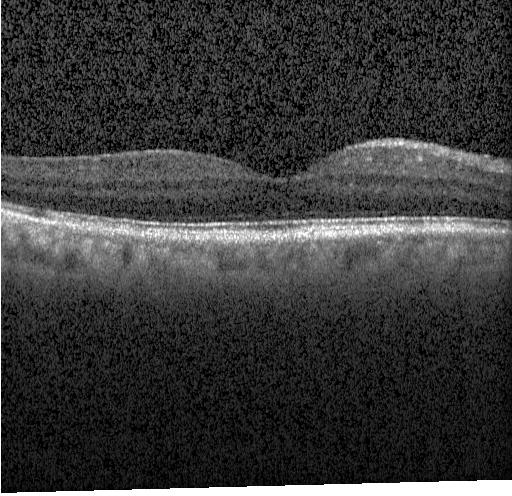

OCT line scan · SD-OCT. No CNV, no DME, and no drusen.